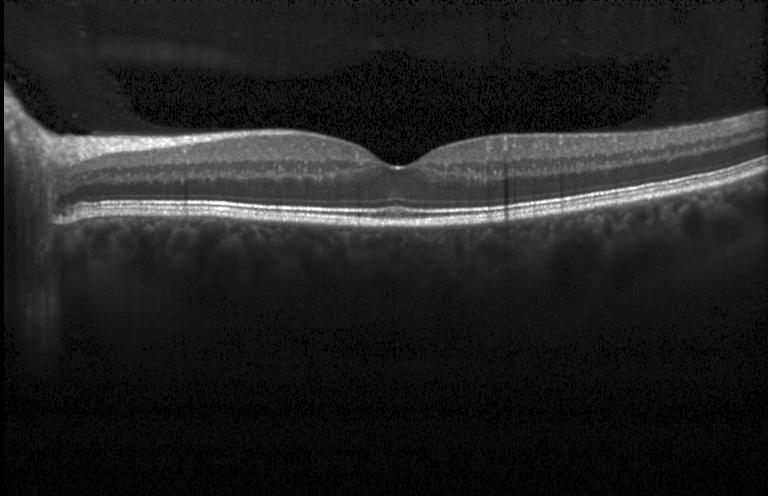 Retinal OCT cross-section; spectral-domain optical coherence tomography — Impression: neither CNV, DME, nor drusen.